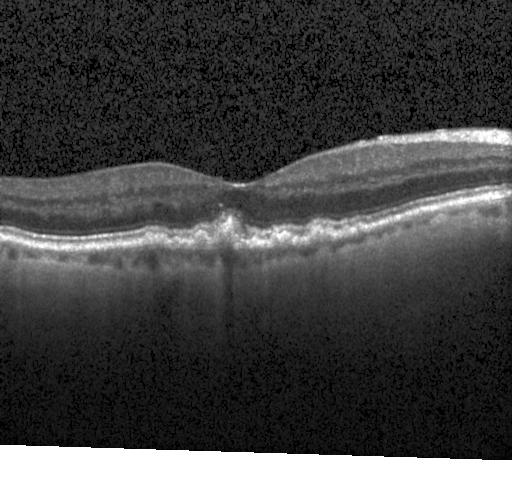
OCT B-scan. Finding: sub-RPE drusenoid deposits.